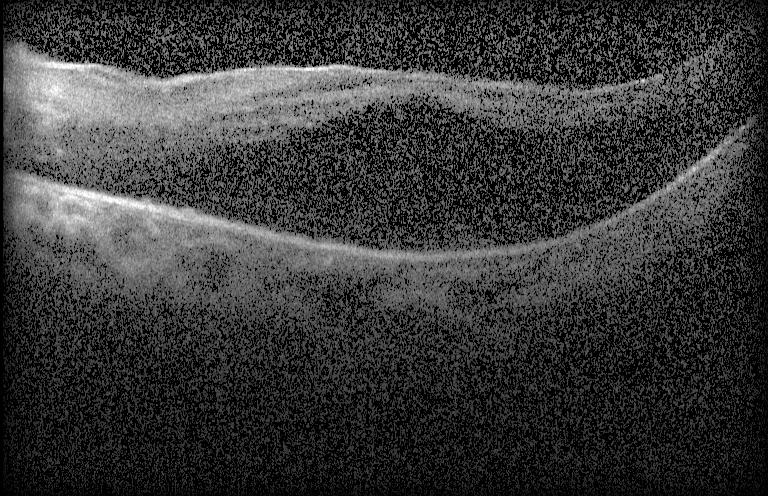
Retinal OCT B-scan. Spectral-domain OCT. Diagnosis: diabetic macular edema (DME).